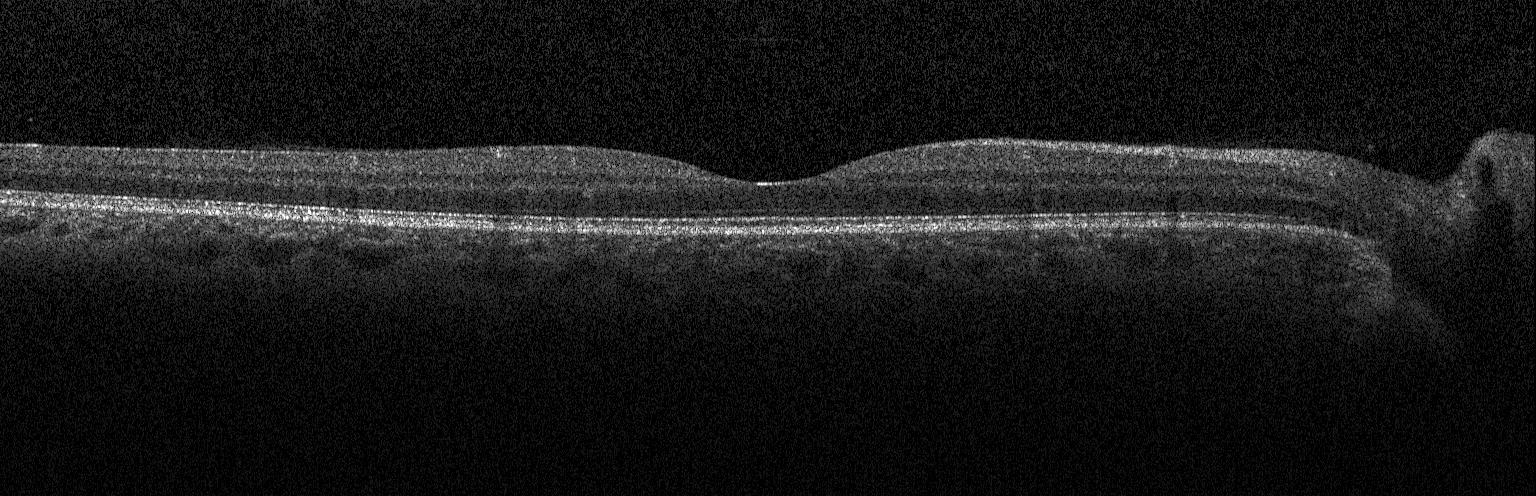 Retinal OCT cross-section
Diagnosis: neither CNV, DME, nor drusen.